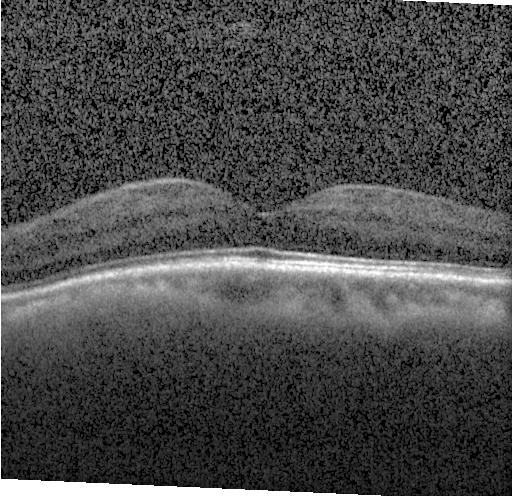 Retinal OCT B-scan. Impression: no choroidal neovascularization, diabetic macular edema, or drusen.